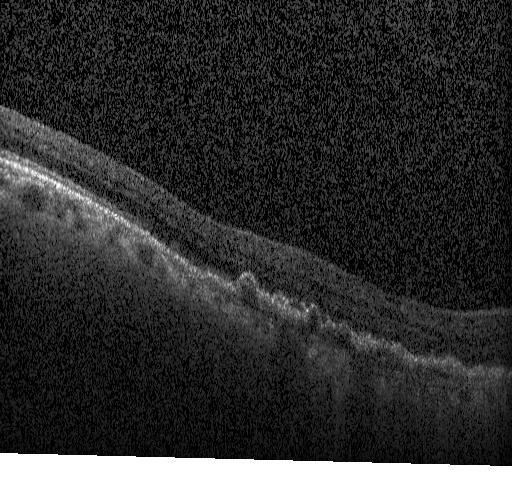
Impression: a choroidal neovascular membrane.